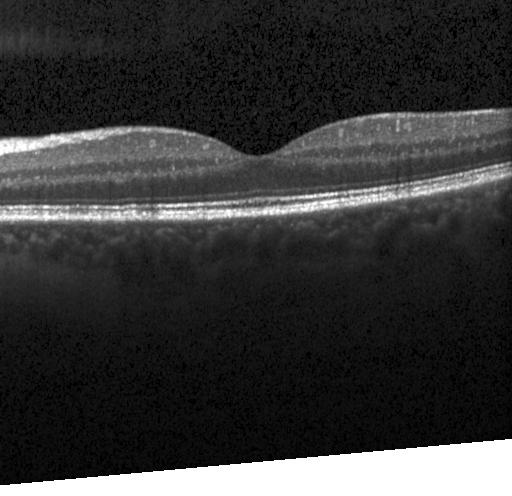 Retinal OCT cross-section; spectral-domain OCT — Macular OCT: no choroidal neovascularization, no diabetic macular edema, and no drusen.